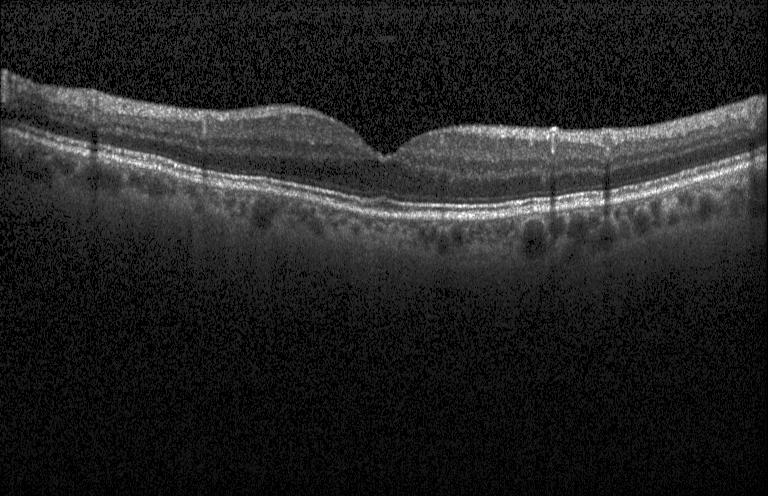
Retinal OCT cross-section · spectral-domain OCT.
The scan shows no choroidal neovascularization, no diabetic macular edema, and no drusen.